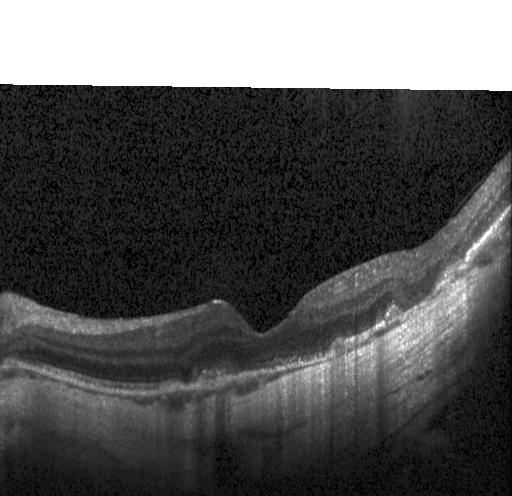
OCT line scan.
Finding: a choroidal neovascular membrane.